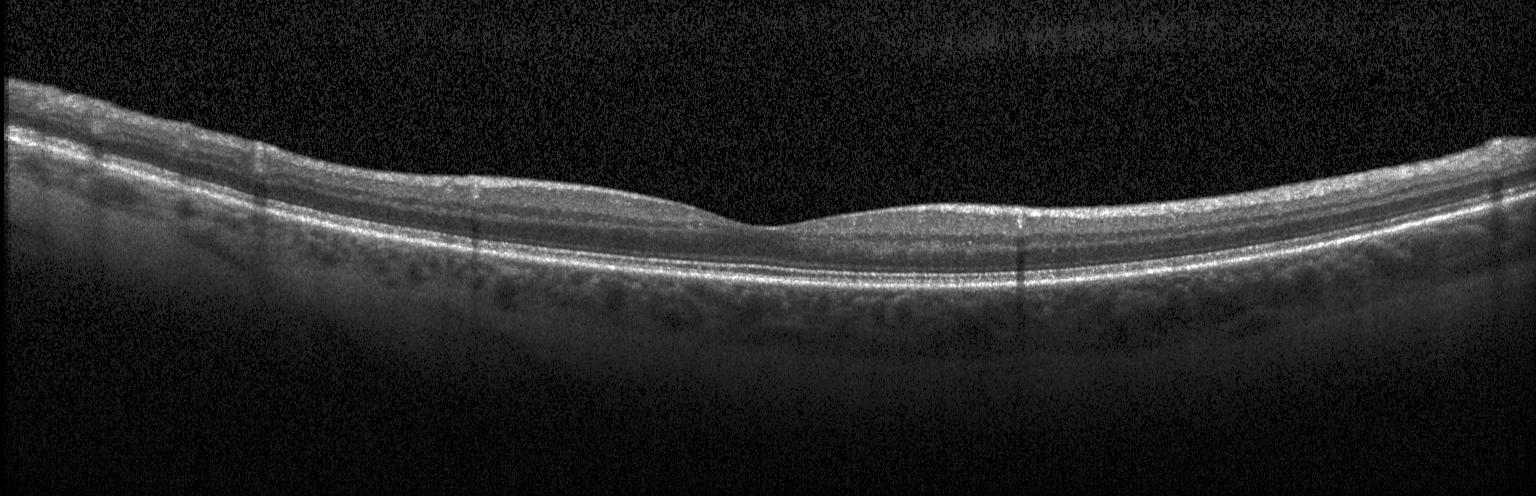

Centered on the fovea. Optical coherence tomography scan. Acquired on a Heidelberg Spectralis. No choroidal neovascularization, diabetic macular edema, or drusen.